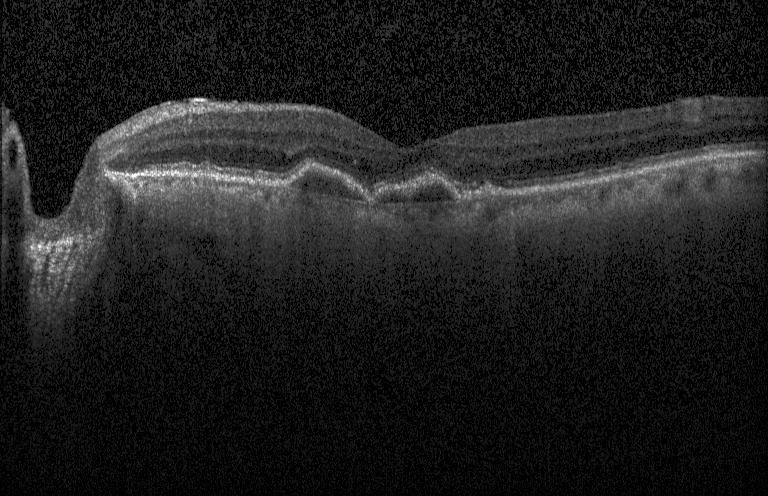 This B-scan demonstrates a choroidal neovascular membrane.